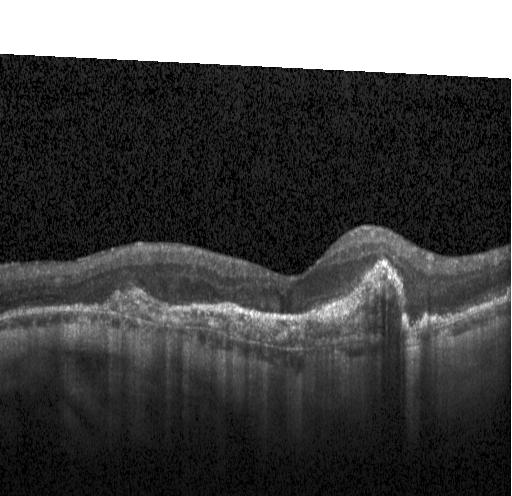

Acquired on a Heidelberg Spectralis. OCT B-scan. Fovea-centered. Macular OCT: a choroidal neovascular membrane.